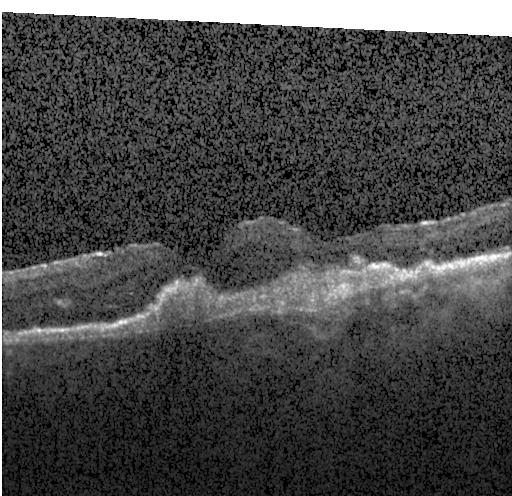 Optical coherence tomography B-scan; acquired on a Heidelberg Spectralis; spectral-domain optical coherence tomography; fovea-centered. Assessment: choroidal neovascularization.